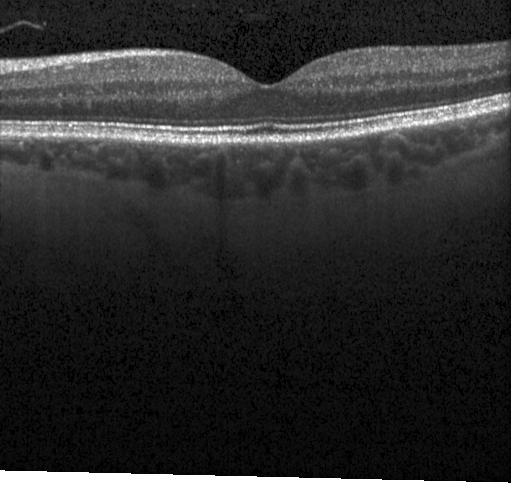
Spectral-domain optical coherence tomography, retinal OCT cross-section — Macular OCT: no choroidal neovascularization, no diabetic macular edema, and no drusen.